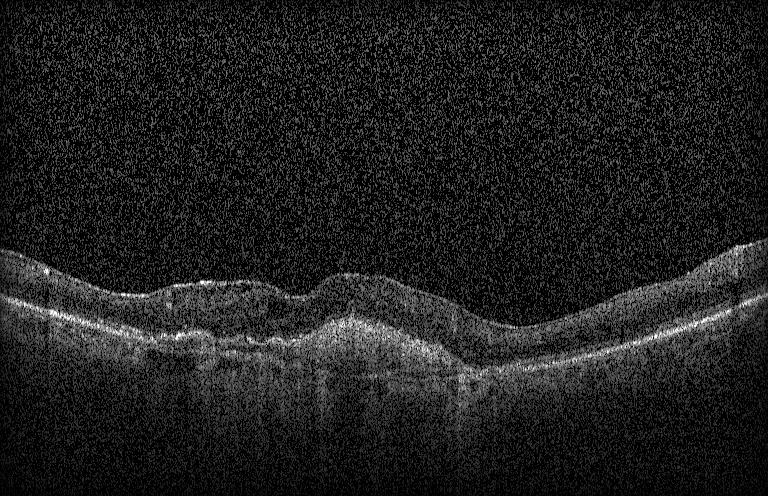

This B-scan demonstrates a choroidal neovascular membrane.